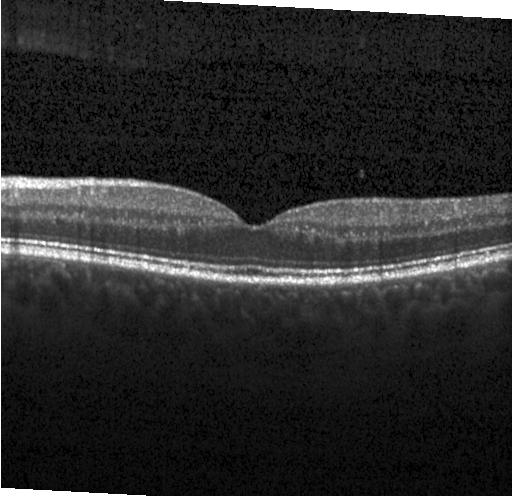 Diagnosis: no evidence of choroidal neovascularization, diabetic macular edema, or drusen.